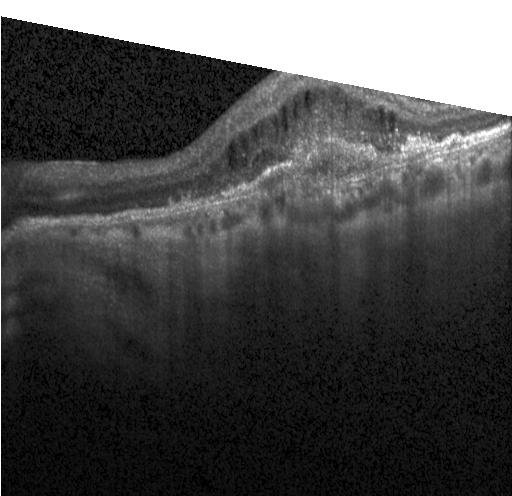 Heidelberg Spectralis OCT system, horizontal scan through the fovea, OCT B-scan. Dx: choroidal neovascularization (CNV).